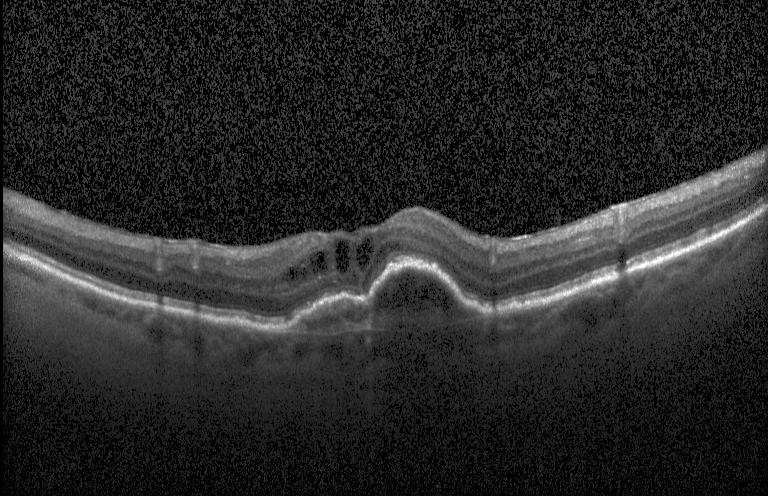
Diagnosis: CNV.